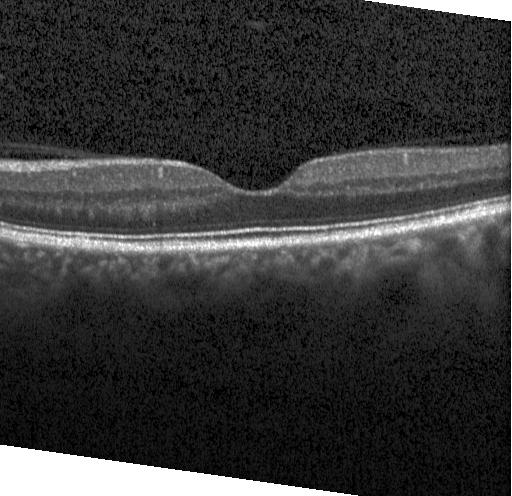

No evidence of CNV, DME, or drusen.